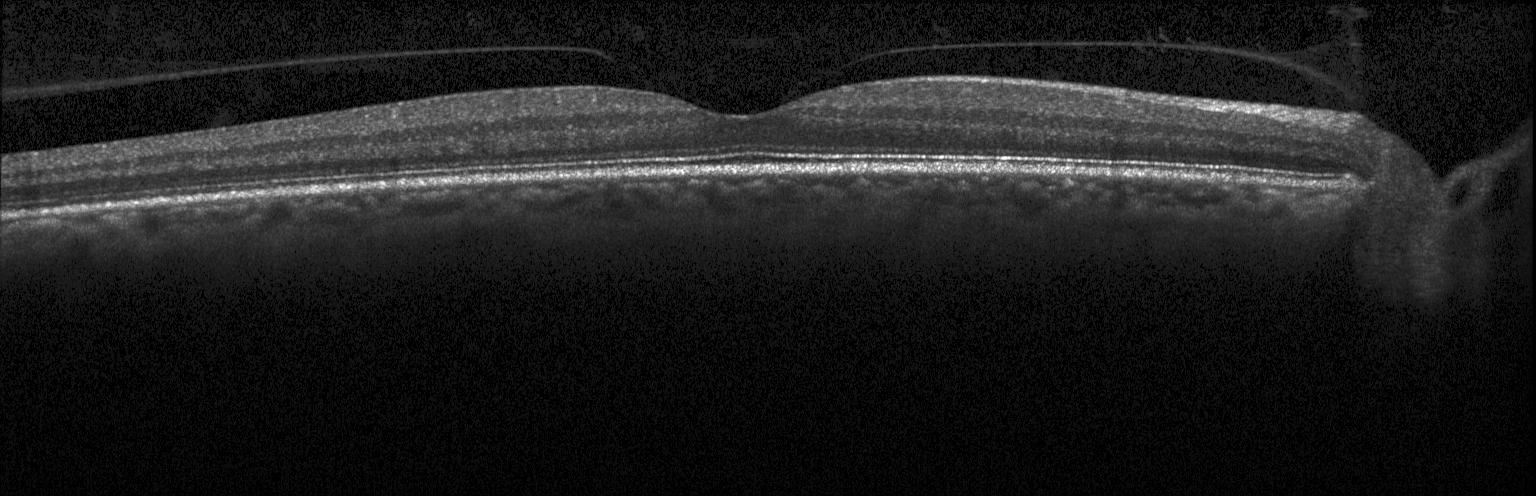 Acquired on a Heidelberg Spectralis, fovea-centered, optical coherence tomography scan, SD-OCT. Impression: no choroidal neovascularization, diabetic macular edema, or drusen.